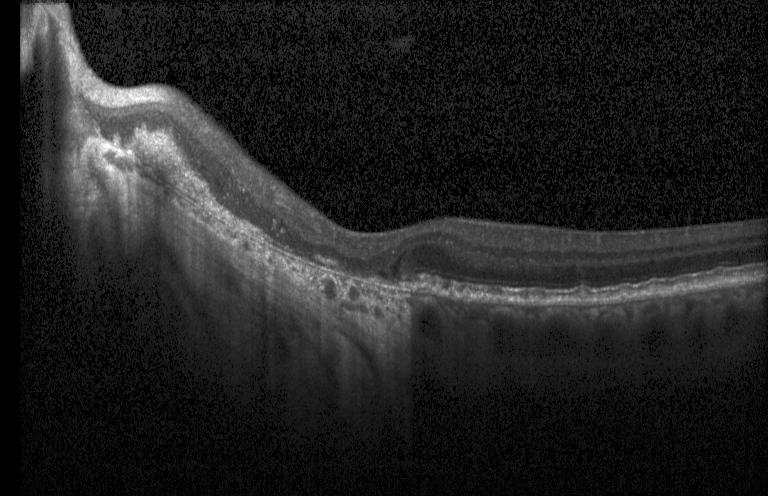 Optical coherence tomography B-scan. Finding: choroidal neovascularization.